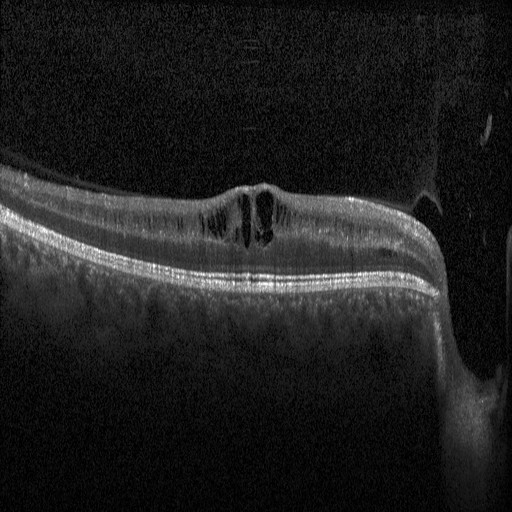

Instrument: Heidelberg Spectralis, SD-OCT, OCT B-scan
The scan shows diabetic macular edema (DME).